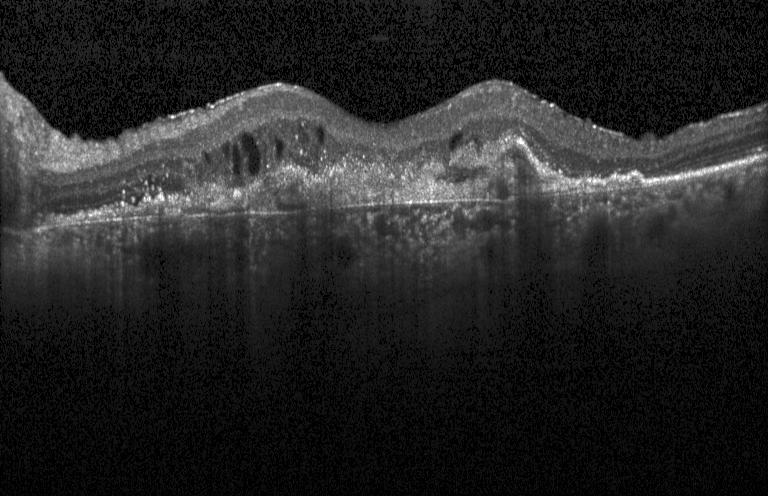

OCT finding: CNV.